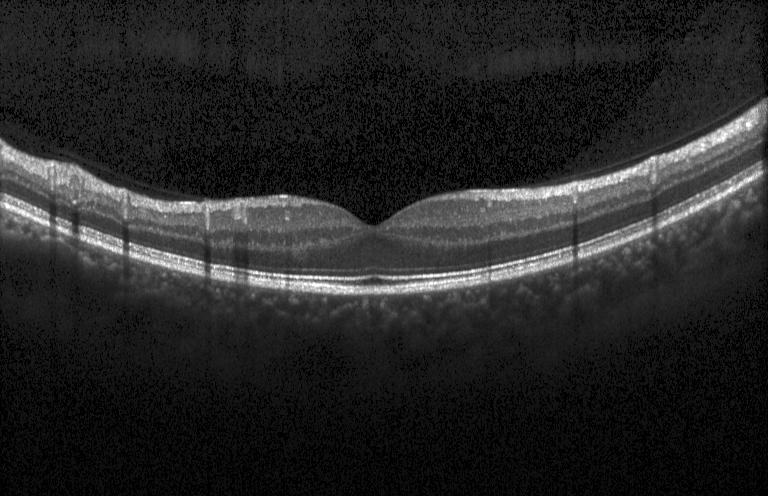

OCT scan showing no choroidal neovascularization, diabetic macular edema, or drusen.